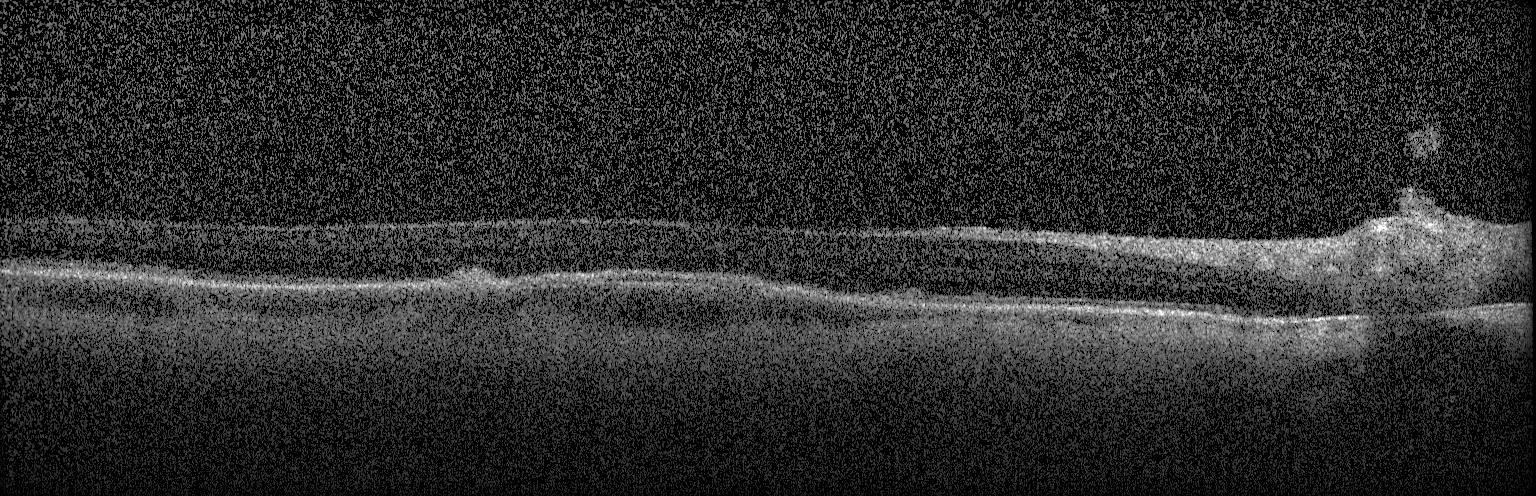

Finding: choroidal neovascularization (CNV).